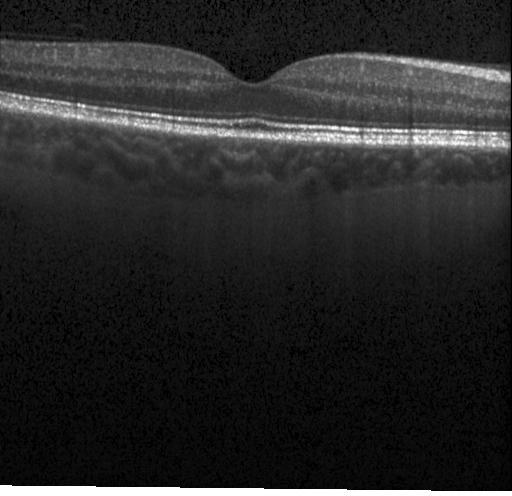

Optical coherence tomography scan. Finding: neither CNV, DME, nor drusen.